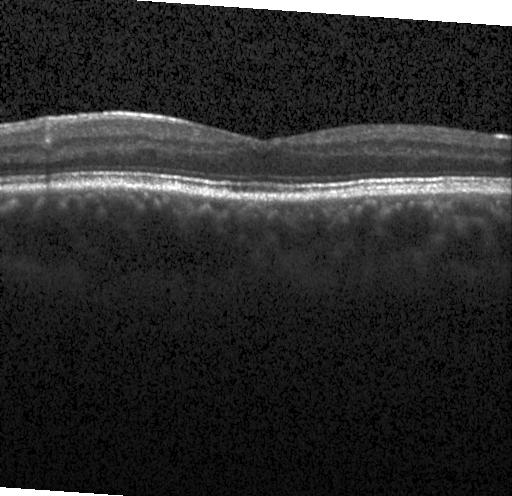

Spectral-domain optical coherence tomography · optical coherence tomography B-scan
Dx: no evidence of CNV, DME, or drusen.